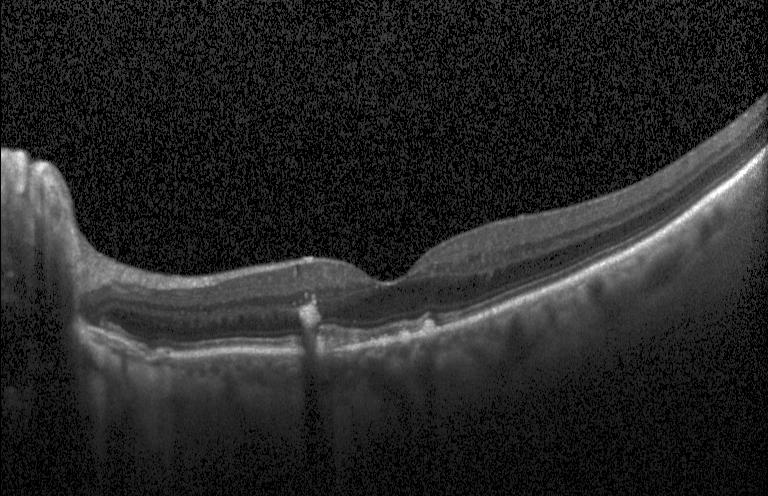 Macular scan; SD-OCT; optical coherence tomography scan — This B-scan demonstrates multiple drusen.